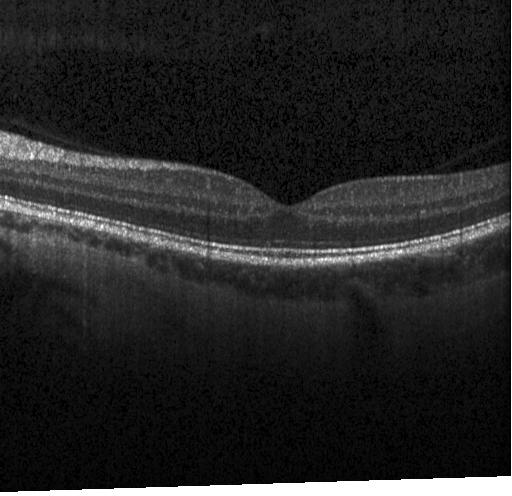 Retinal OCT cross-section. No choroidal neovascularization, no diabetic macular edema, and no drusen.